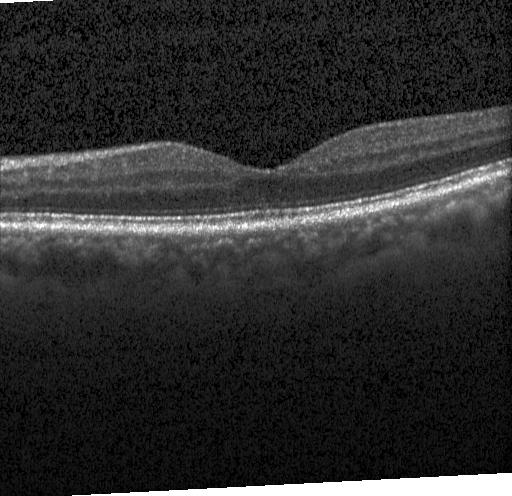
Acquired on a Heidelberg Spectralis. Fovea-centered. Spectral-domain optical coherence tomography. OCT B-scan. Impression: no evidence of CNV, DME, or drusen.